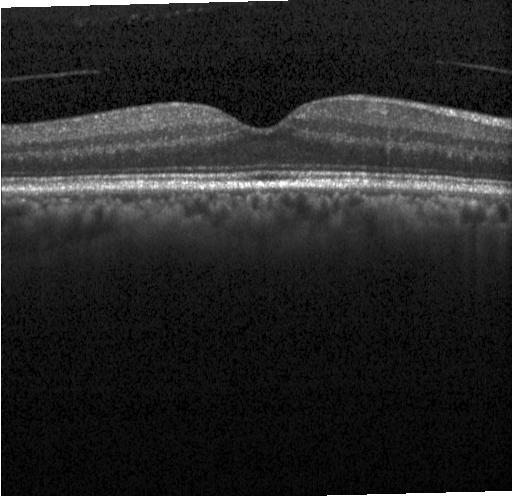

The scan shows no choroidal neovascularization, no diabetic macular edema, and no drusen.